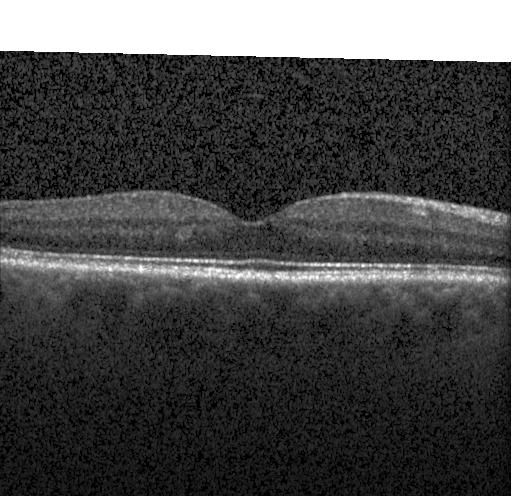 OCT finding: neither CNV, DME, nor drusen.